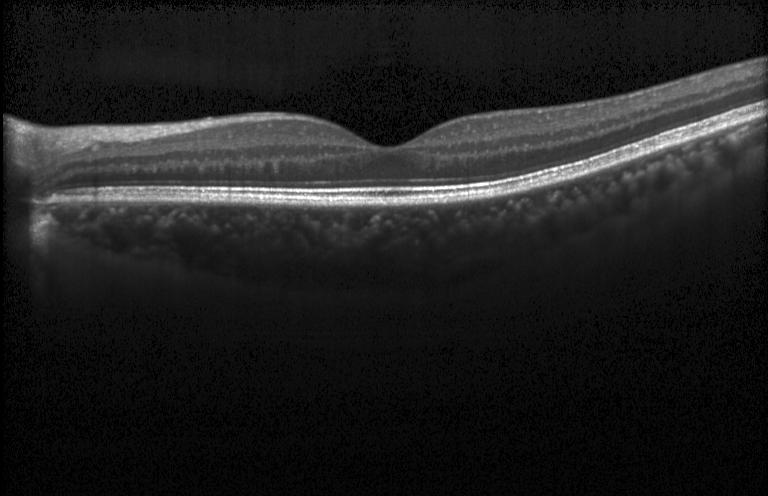
Spectral-domain OCT · instrument: Heidelberg Spectralis · macular scan · optical coherence tomography scan
Assessment: no evidence of CNV, DME, or drusen.